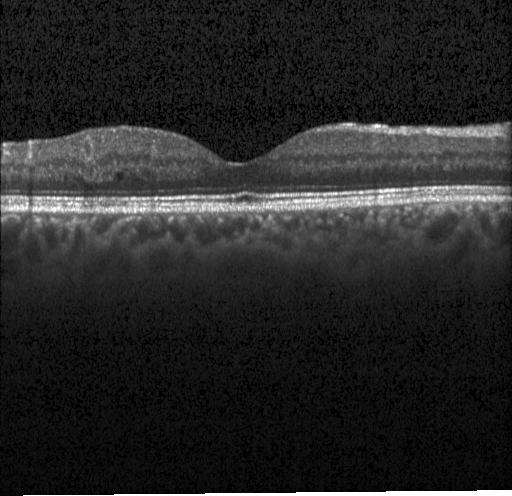 Fovea-centered; Heidelberg Spectralis OCT system; optical coherence tomography scan — The scan shows DME.